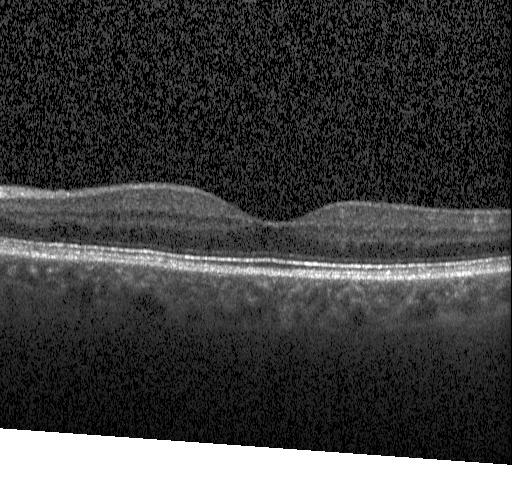 Instrument: Heidelberg Spectralis; retinal OCT cross-section; spectral-domain OCT; centered on the fovea — Dx: no CNV, no DME, and no drusen.